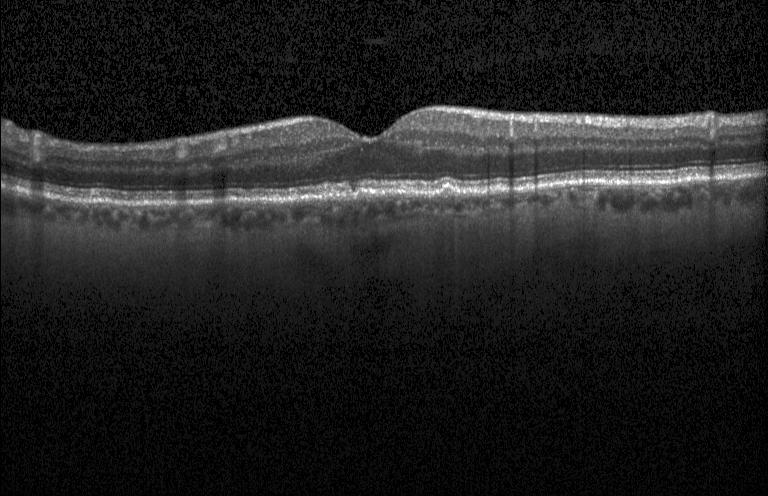
This B-scan demonstrates drusen.